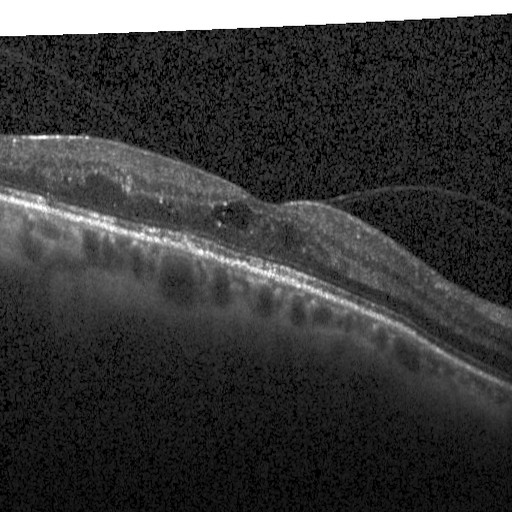 Finding: diabetic macular edema (DME).